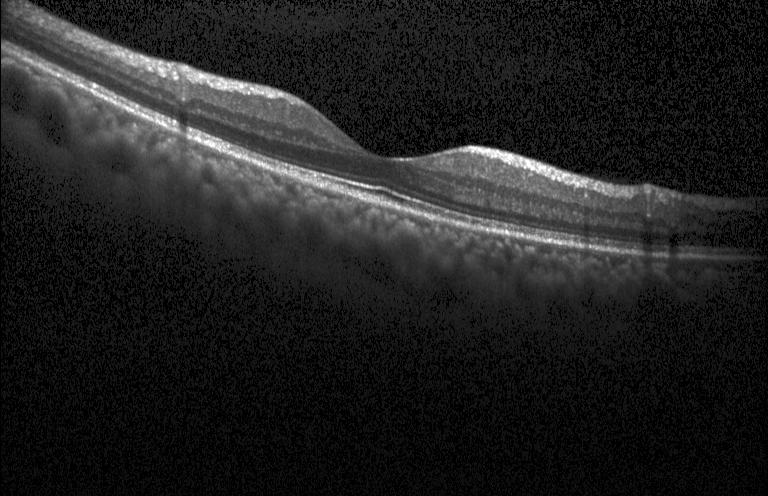

Instrument: Heidelberg Spectralis, optical coherence tomography scan, through the macula, spectral-domain optical coherence tomography. Assessment: no choroidal neovascularization, no diabetic macular edema, and no drusen.